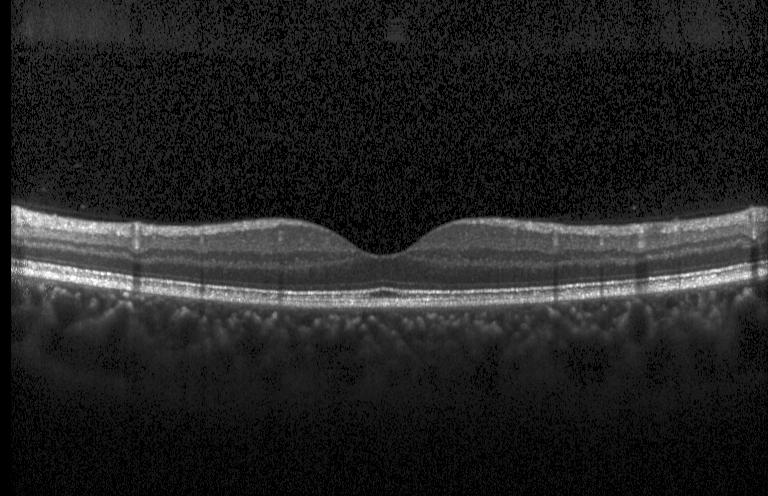
Horizontal scan through the fovea, acquired on a Heidelberg Spectralis, spectral-domain OCT, optical coherence tomography B-scan — Impression: neither CNV, DME, nor drusen.